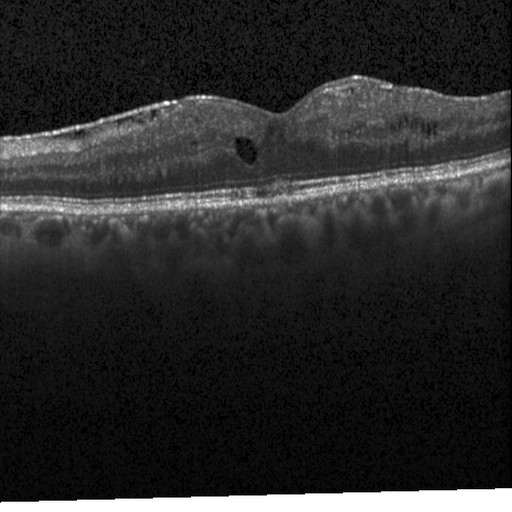

Optical coherence tomography scan. Horizontal scan through the fovea. Heidelberg Spectralis OCT system. Spectral-domain OCT. Macular OCT: diabetic macular edema.